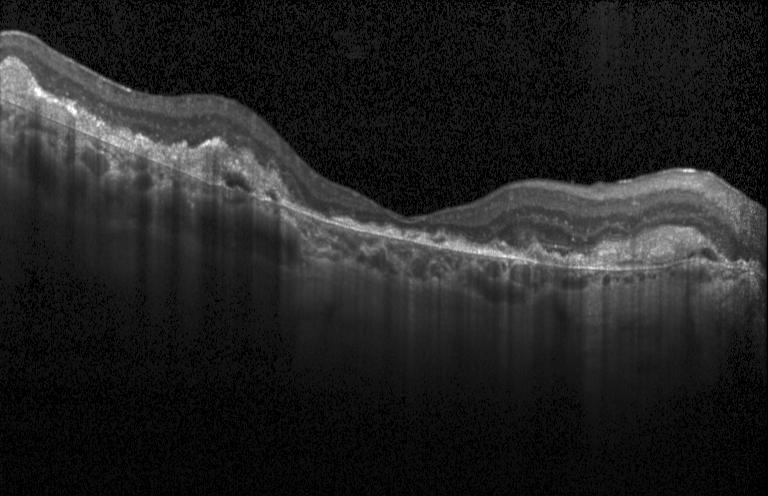 Diagnosis: a choroidal neovascular membrane.